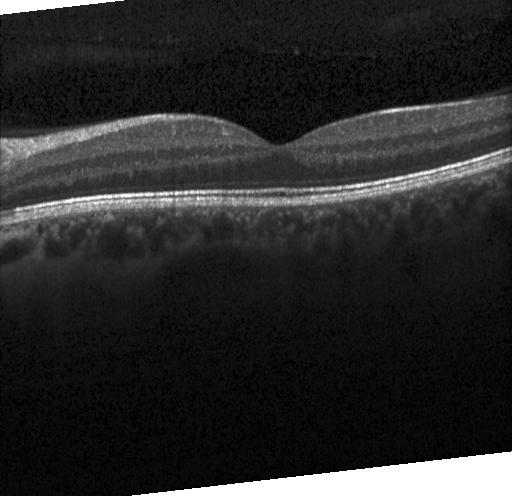

OCT line scan — Finding: no choroidal neovascularization, diabetic macular edema, or drusen.